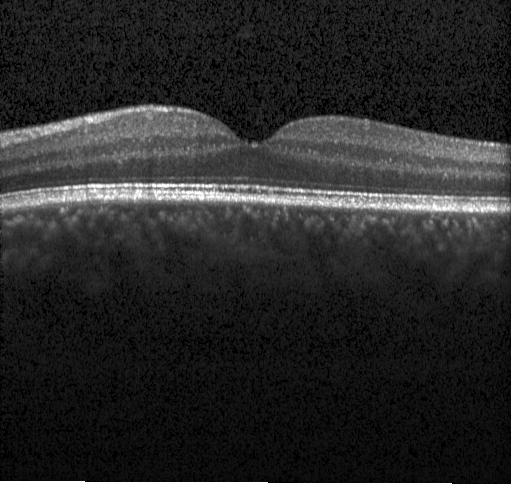
Macular OCT demonstrating no choroidal neovascularization, diabetic macular edema, or drusen.